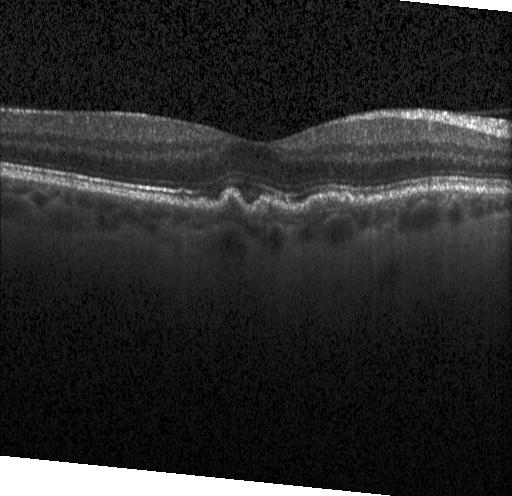 Acquired on a Heidelberg Spectralis; spectral-domain optical coherence tomography; optical coherence tomography B-scan.
Macular OCT: sub-RPE drusenoid deposits.